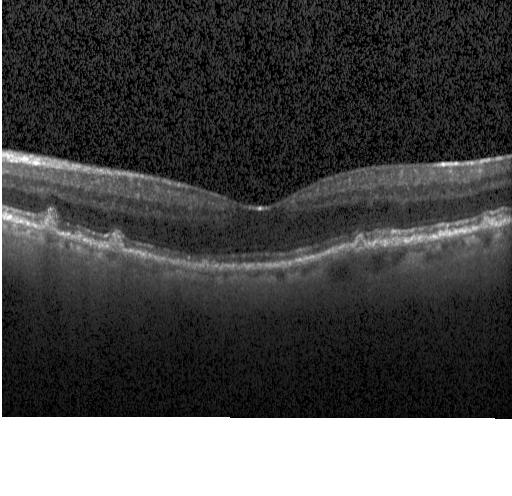 Optical coherence tomography B-scan · Heidelberg Spectralis · macular scan
OCT finding: sub-RPE drusenoid deposits.